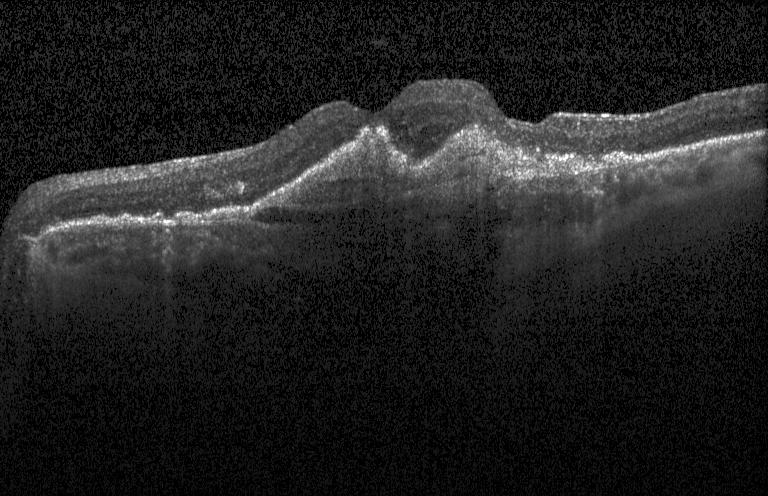

Optical coherence tomography scan. Finding: a choroidal neovascular membrane.